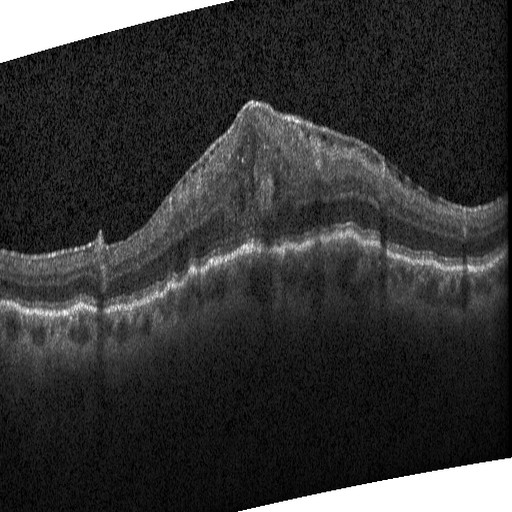
Impression: diabetic macular edema (DME).